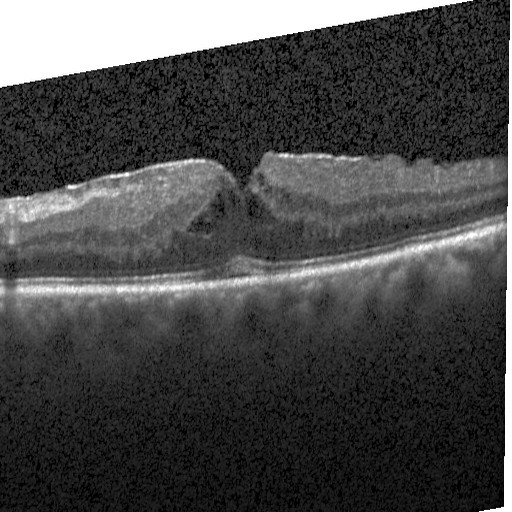 Spectral-domain OCT B-scan: diabetic macular edema (DME).